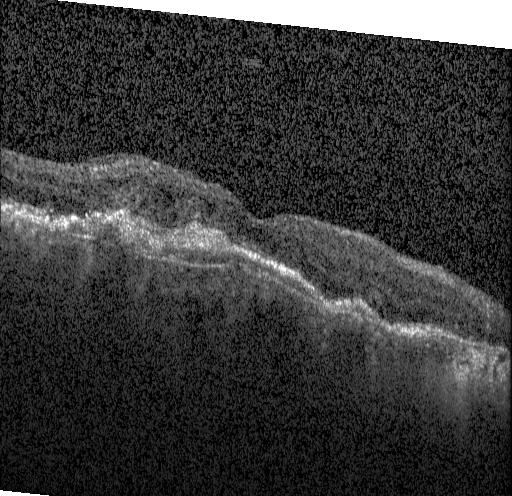 OCT B-scan · centered on the fovea · acquired on a Heidelberg Spectralis. A choroidal neovascular membrane.